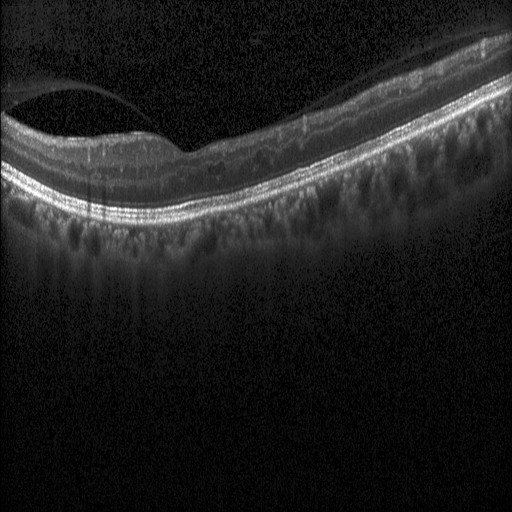
Assessment: DME.